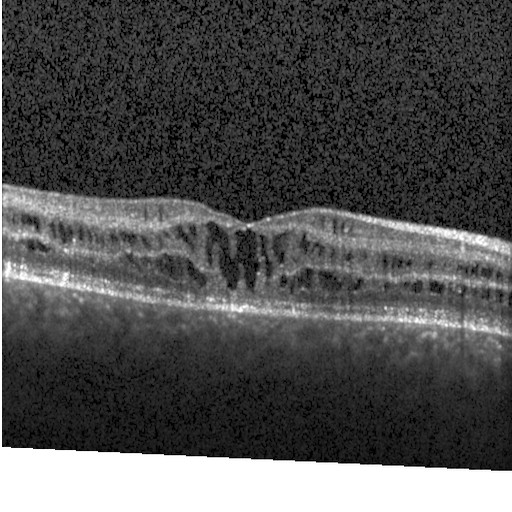
Acquired on a Heidelberg Spectralis · OCT line scan · SD-OCT · centered on the fovea.
This B-scan demonstrates diabetic macular edema.